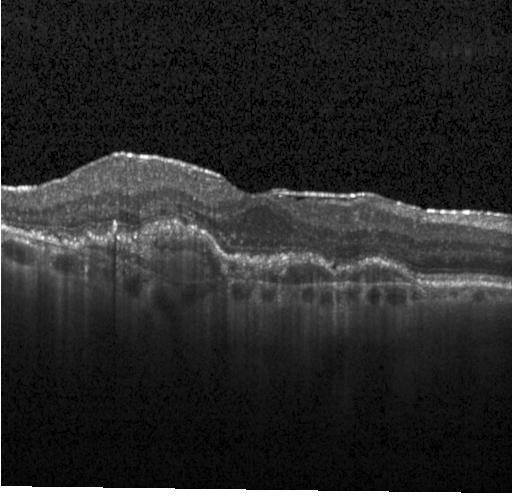
This B-scan demonstrates a choroidal neovascular membrane.